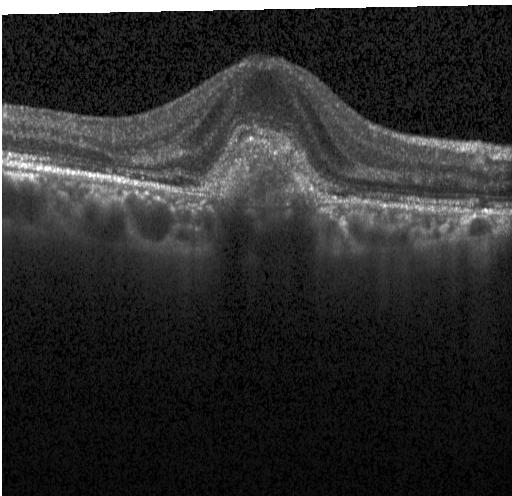
Dx: a choroidal neovascular membrane.